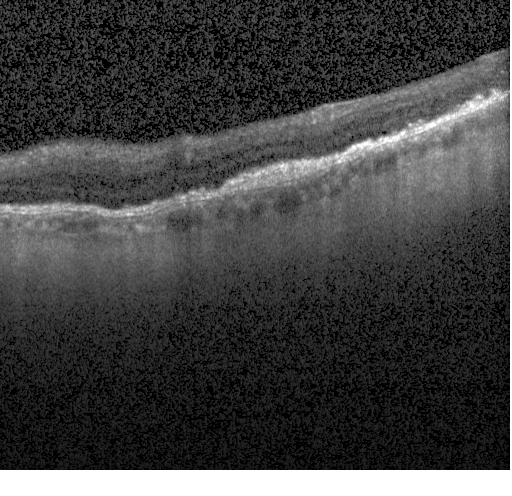
Heidelberg Spectralis · OCT line scan · through the macula · SD-OCT — Finding: a choroidal neovascular membrane.